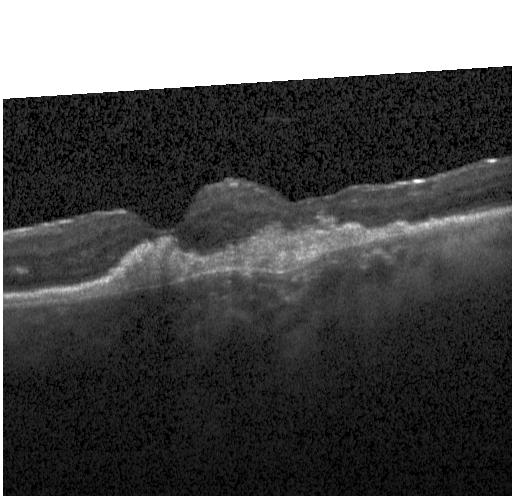
Finding: choroidal neovascularization (CNV).